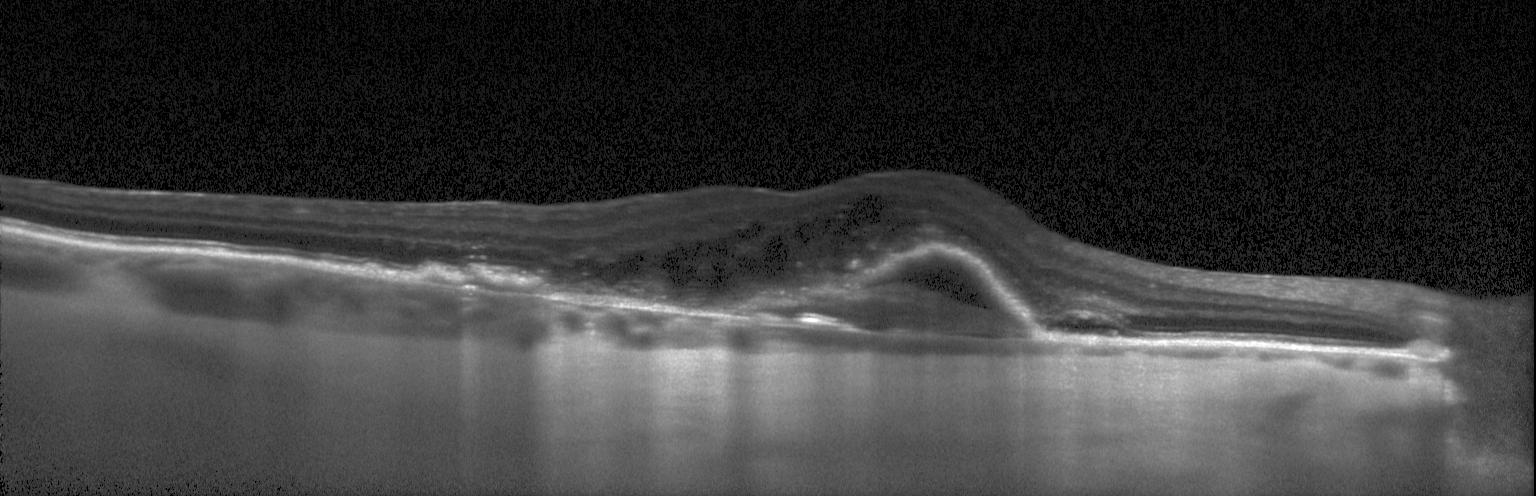 Retinal OCT cross-section. Macular OCT: a choroidal neovascular membrane.